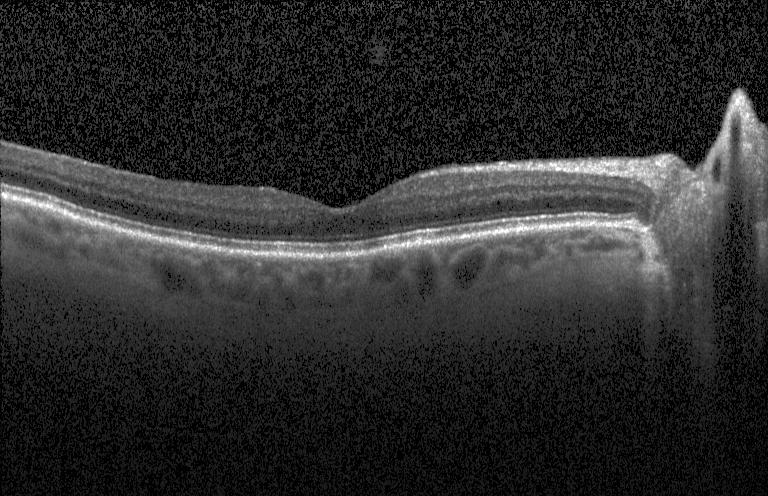 Finding: no evidence of choroidal neovascularization, diabetic macular edema, or drusen.